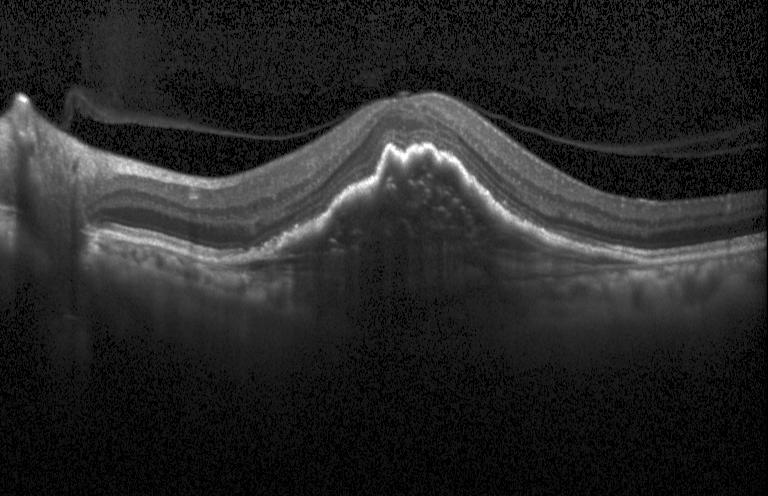
OCT line scan.
Impression: CNV.